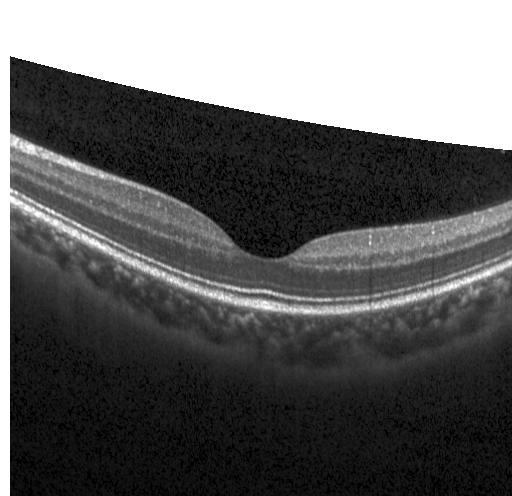 Macular OCT: no evidence of CNV, DME, or drusen.